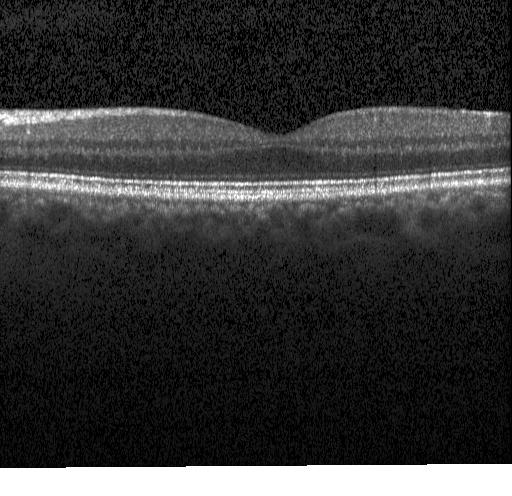 Retinal OCT B-scan. Macular scan.
Impression: no choroidal neovascularization, no diabetic macular edema, and no drusen.